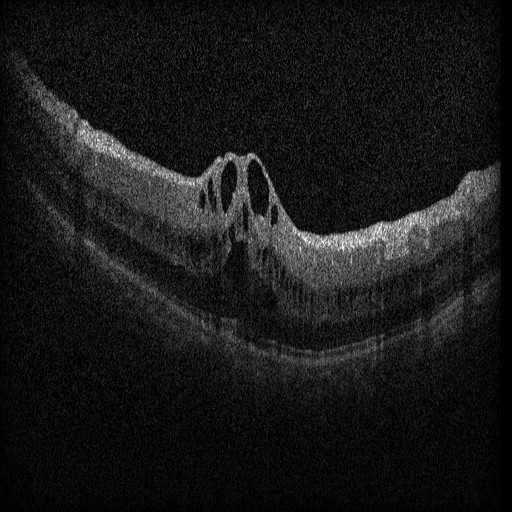
Optical coherence tomography B-scan.
Macular OCT: DME.